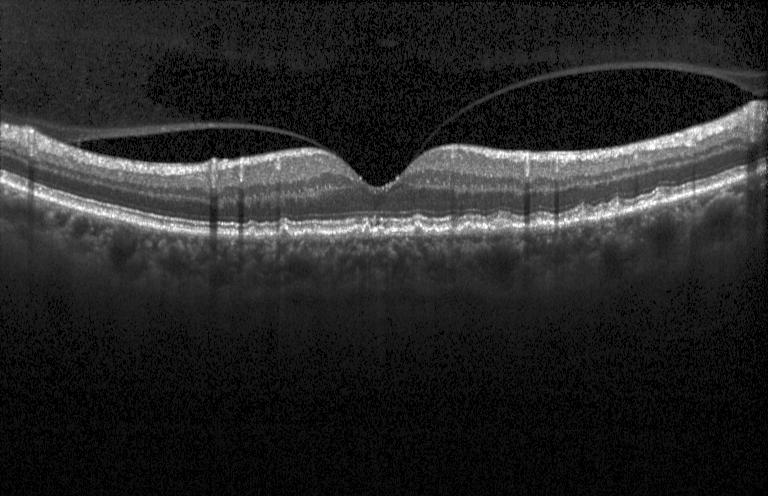 SD-OCT · acquired on a Heidelberg Spectralis · macular scan · optical coherence tomography scan. This B-scan demonstrates multiple drusen.